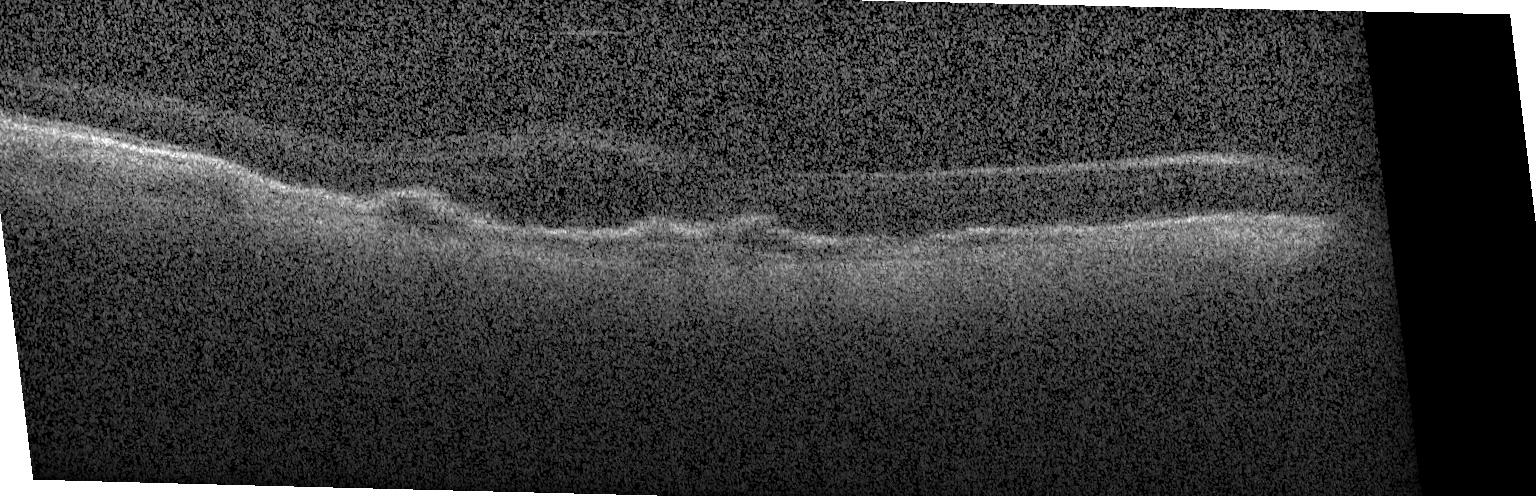
OCT line scan. This B-scan demonstrates a choroidal neovascular membrane.